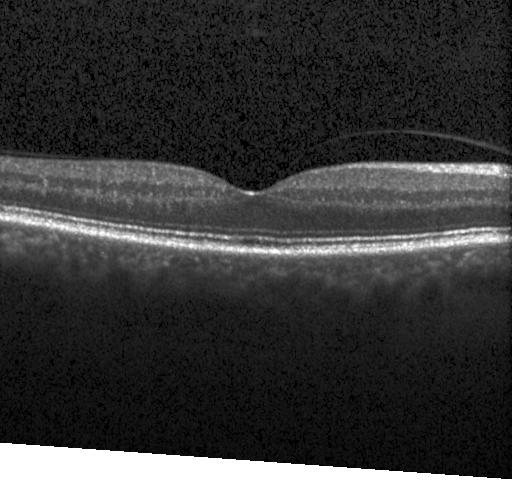

Diagnosis: neither choroidal neovascularization, diabetic macular edema, nor drusen.